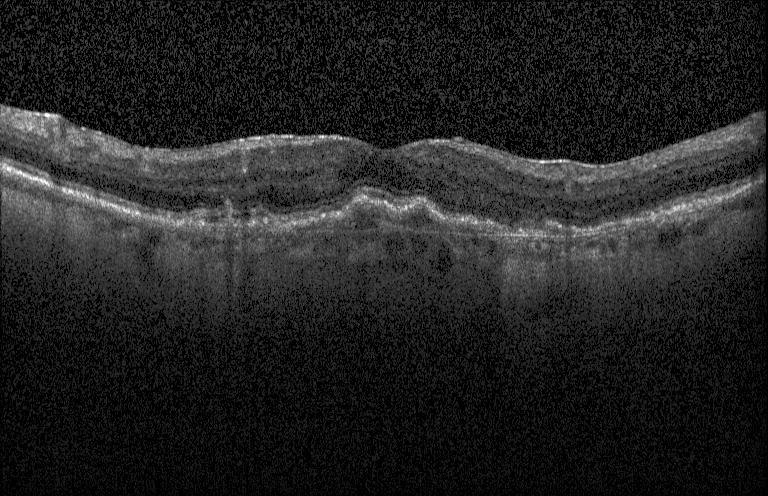 Retinal OCT B-scan
Assessment: choroidal neovascularization.